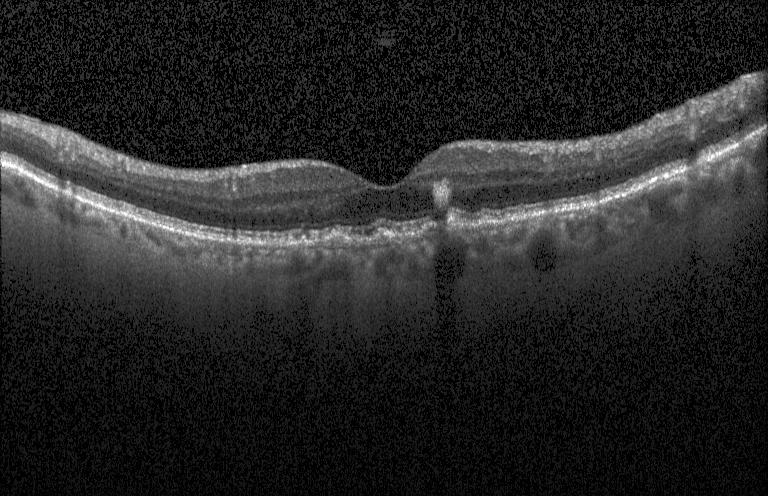 Dx: multiple drusen.